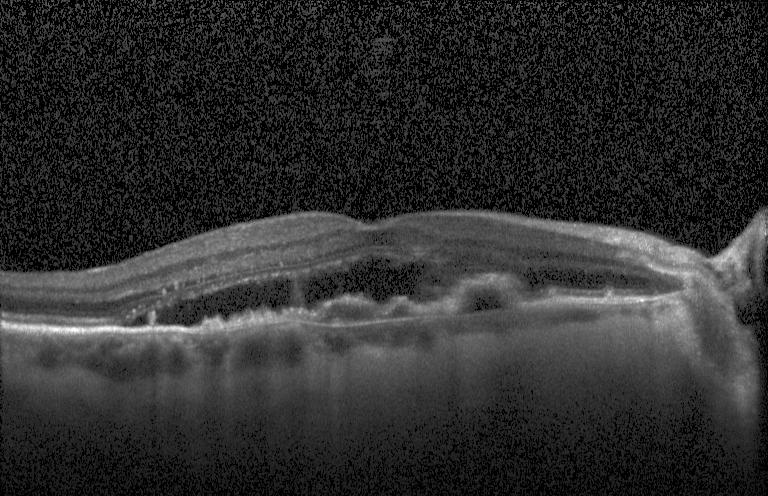

Heidelberg Spectralis OCT system. SD-OCT. Through the macula. OCT B-scan — Dx: a choroidal neovascular membrane.